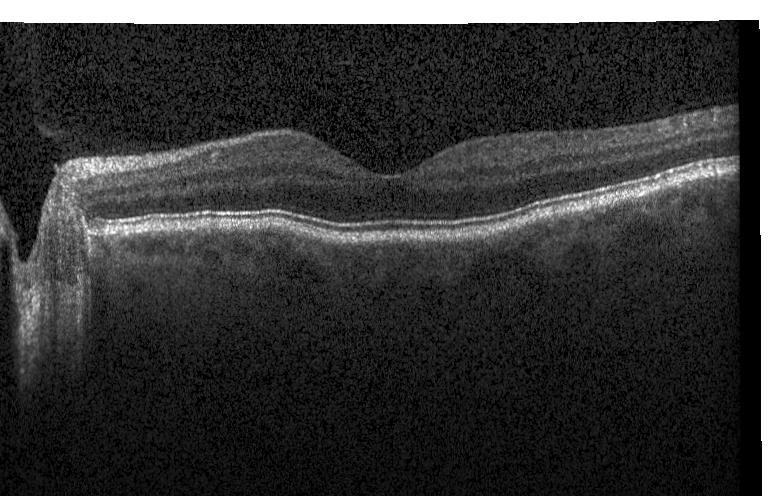 Diagnosis: no choroidal neovascularization, no diabetic macular edema, and no drusen.